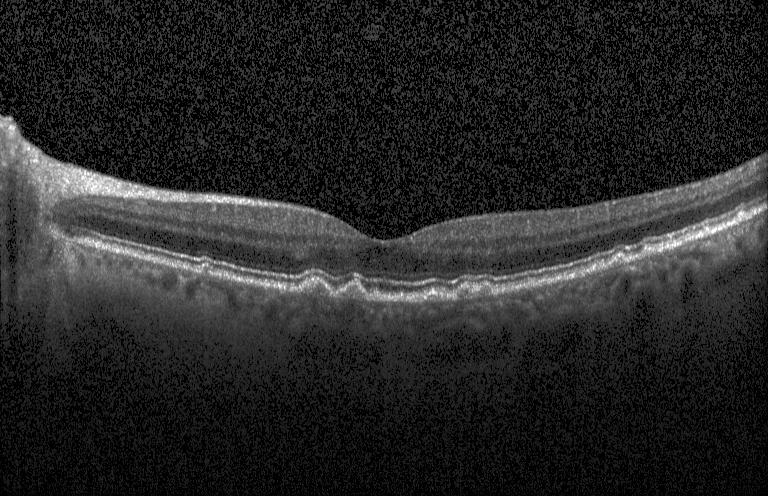

Retinal OCT B-scan. Spectral-domain optical coherence tomography
Finding: drusen.